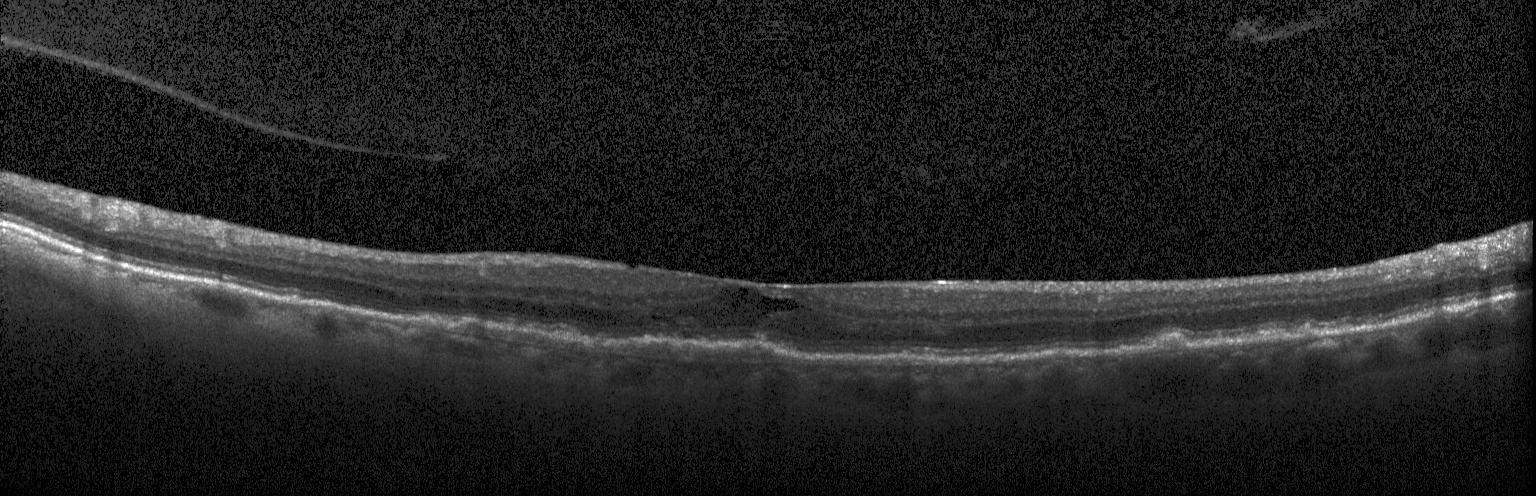 Spectral-domain optical coherence tomography; retinal OCT cross-section.
Impression: choroidal neovascularization (CNV).